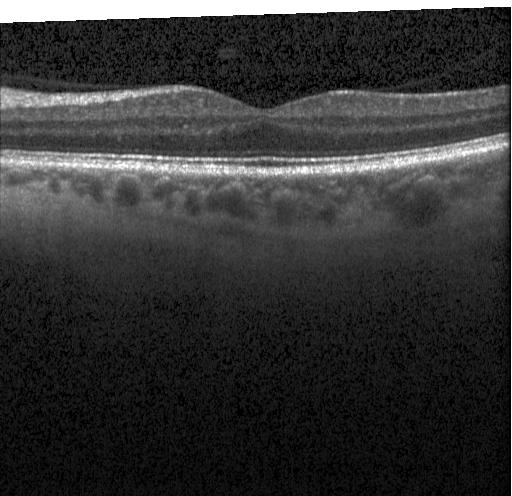
Horizontal scan through the fovea · retinal OCT cross-section
Dx: no evidence of CNV, DME, or drusen.